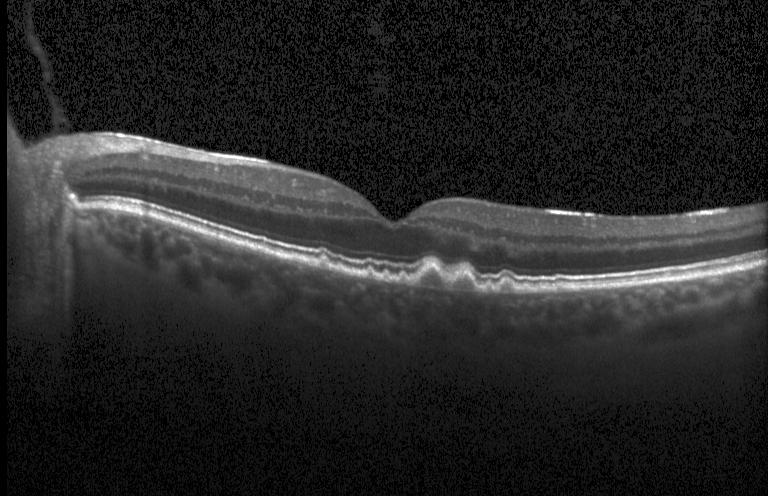 Macular OCT demonstrating drusen.